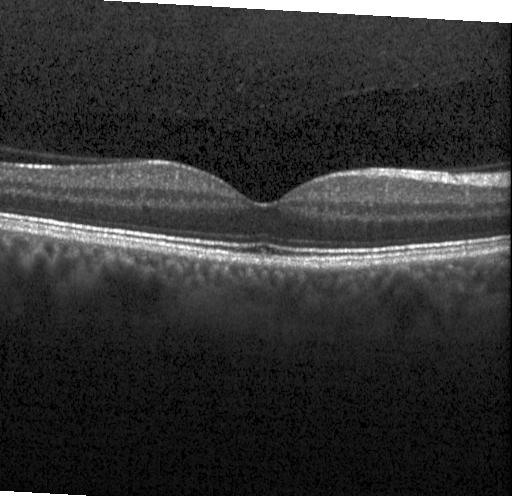
Through the macula · retinal OCT cross-section. Diagnosis: no evidence of CNV, DME, or drusen.